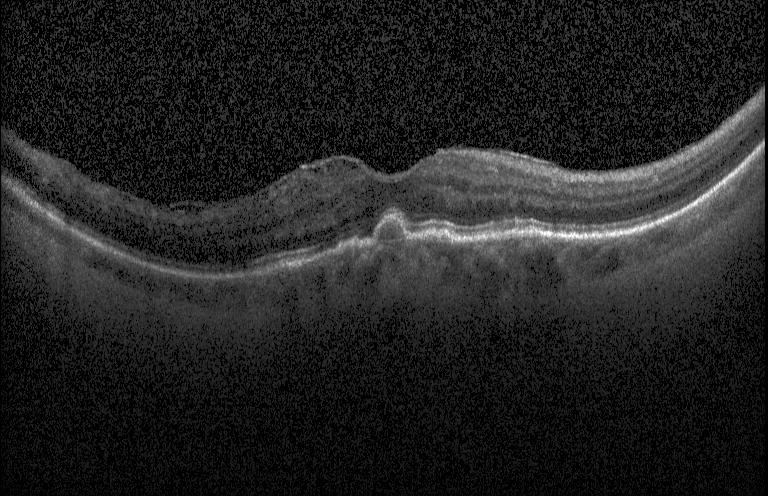

The scan shows multiple drusen.